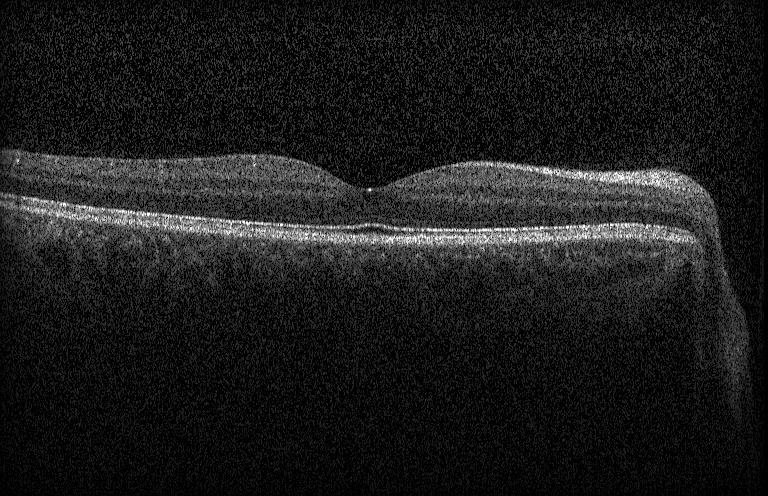
Optical coherence tomography scan. Finding: no choroidal neovascularization, no diabetic macular edema, and no drusen.